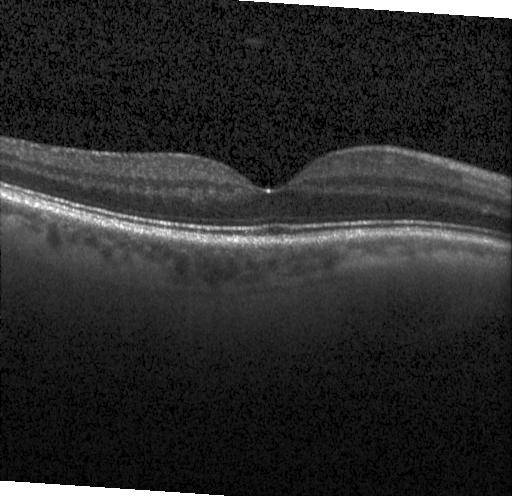
Spectral-domain OCT, OCT B-scan
Finding: no evidence of choroidal neovascularization, diabetic macular edema, or drusen.